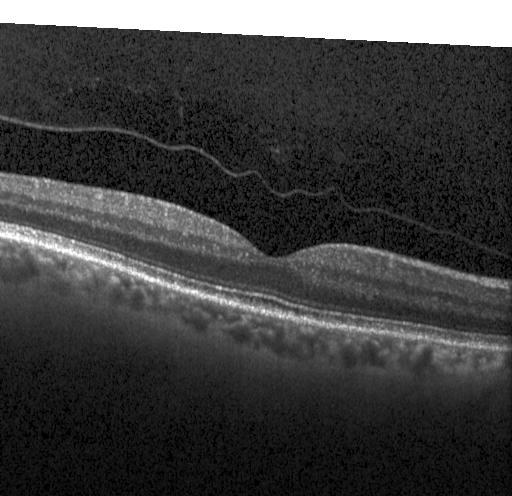
Retinal OCT cross-section. Finding: no choroidal neovascularization, diabetic macular edema, or drusen.